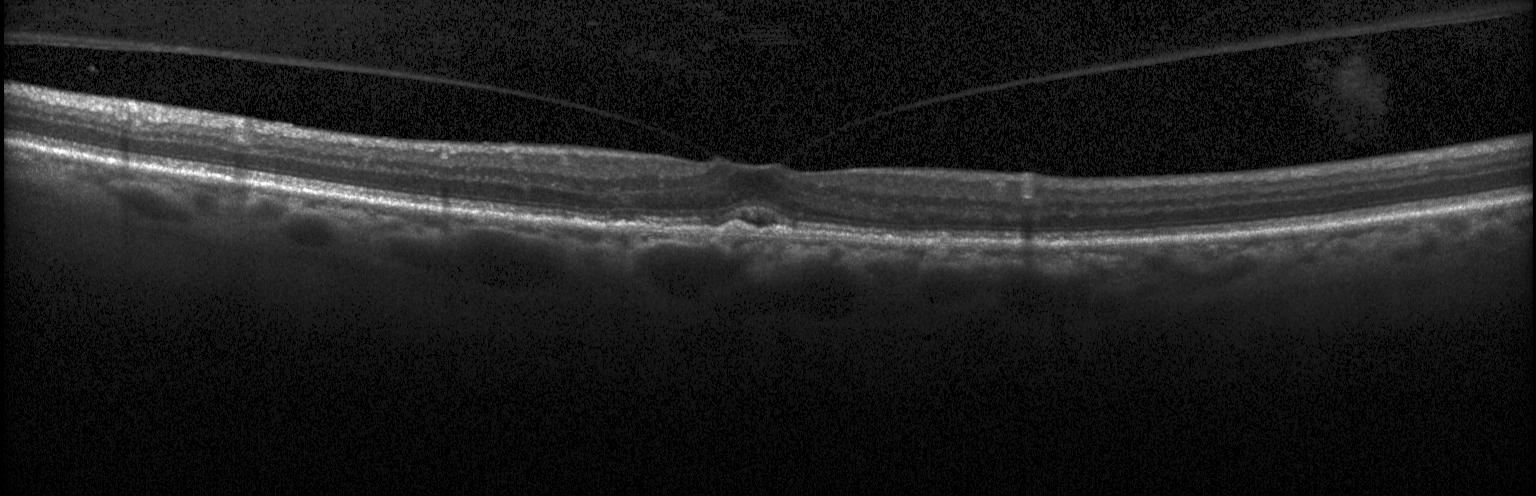 Spectral-domain OCT, OCT B-scan, Heidelberg Spectralis OCT system, centered on the fovea — Diagnosis: choroidal neovascularization.